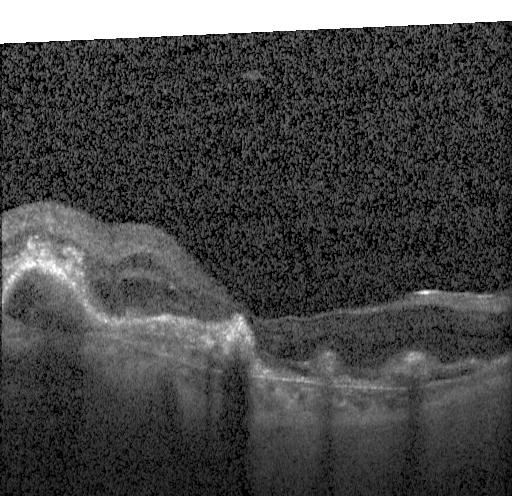 Spectral-domain OCT B-scan: CNV.